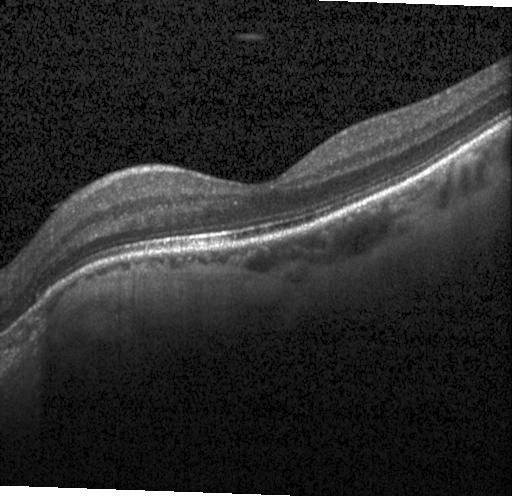 Spectral-domain OCT, OCT B-scan — Diagnosis: neither choroidal neovascularization, diabetic macular edema, nor drusen.